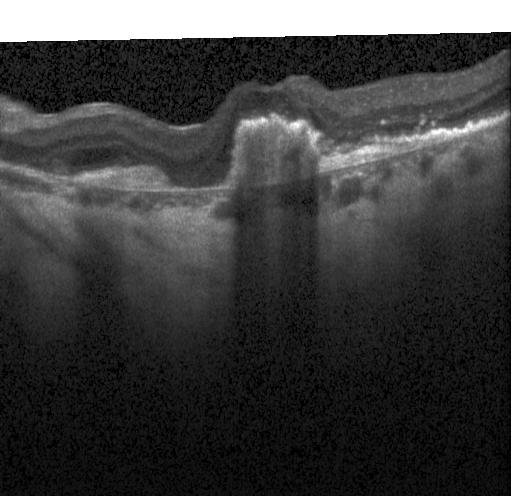 Retinal OCT cross-section showing a choroidal neovascular membrane.